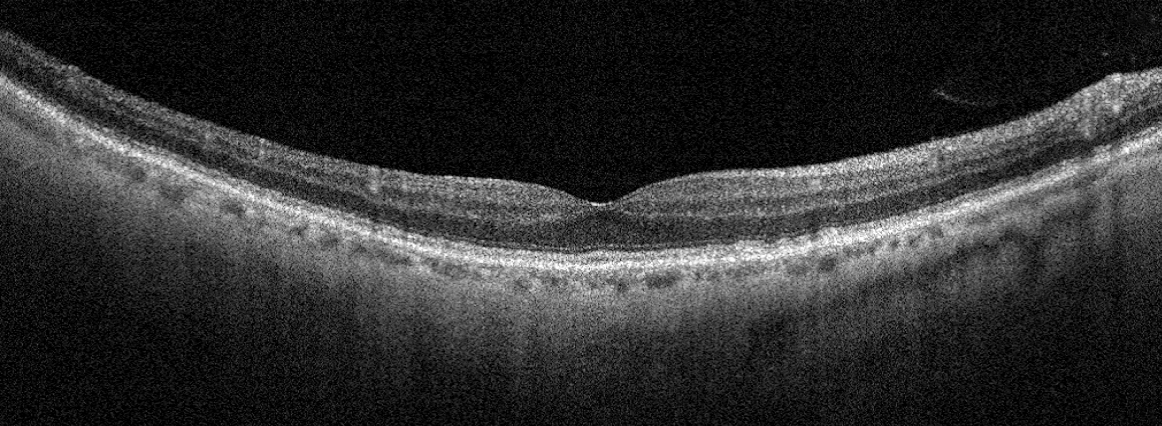 Optovue Avanti RTVue XR. Oculus dexter. Retinal OCT B-scan — Impression: age-related macular degeneration.